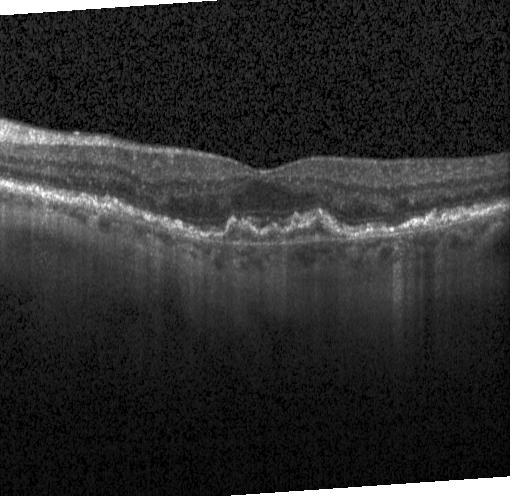

OCT B-scan.
Impression: CNV.